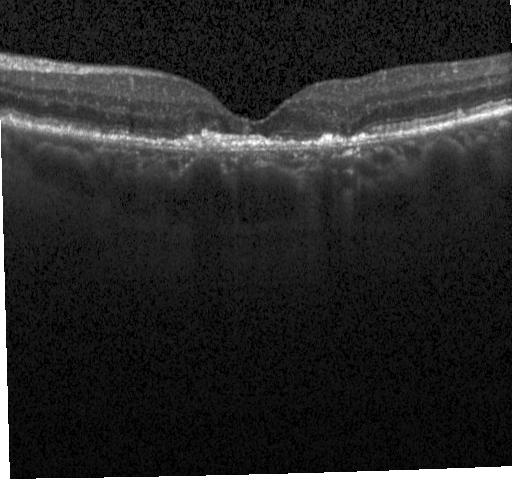 OCT B-scan, SD-OCT, Heidelberg Spectralis OCT system, macular scan. Impression: choroidal neovascularization (CNV).